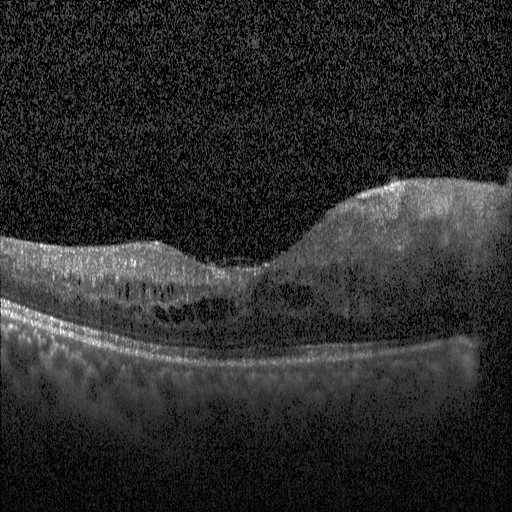
SD-OCT, optical coherence tomography B-scan, Heidelberg Spectralis — Impression: diabetic macular edema.